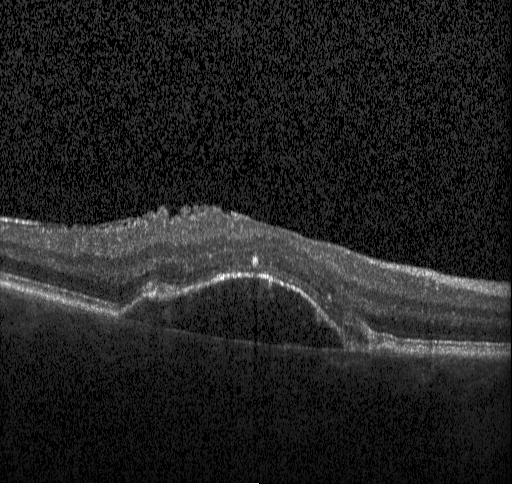
Spectral-domain optical coherence tomography, Heidelberg Spectralis, OCT B-scan, fovea-centered. Diagnosis: a choroidal neovascular membrane.